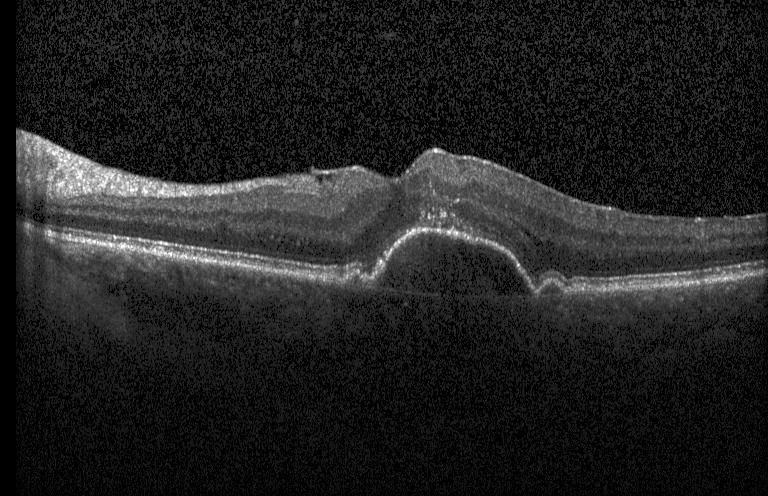
Retinal OCT cross-section showing choroidal neovascularization (CNV).